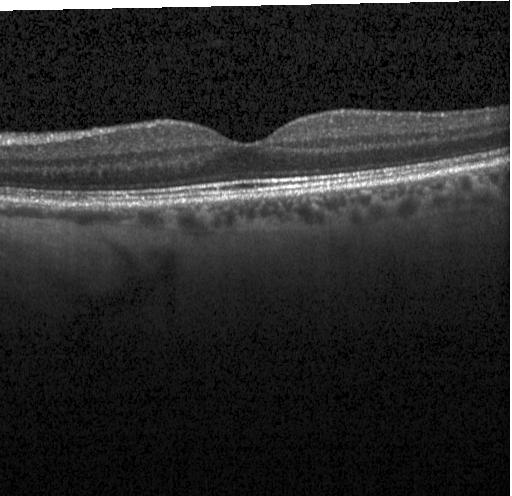
OCT B-scan · horizontal scan through the fovea — This B-scan demonstrates no CNV, DME, or drusen.